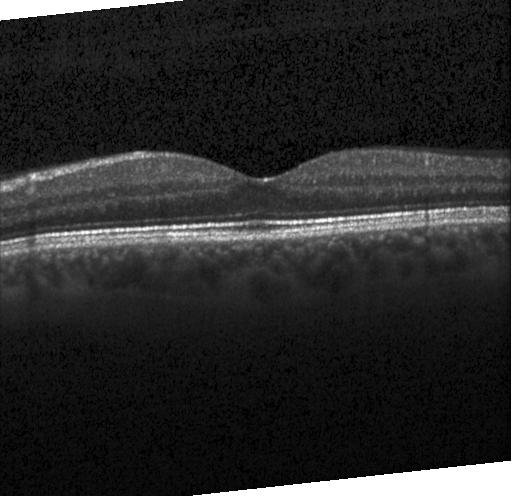

Optical coherence tomography scan — Assessment: no choroidal neovascularization, no diabetic macular edema, and no drusen.